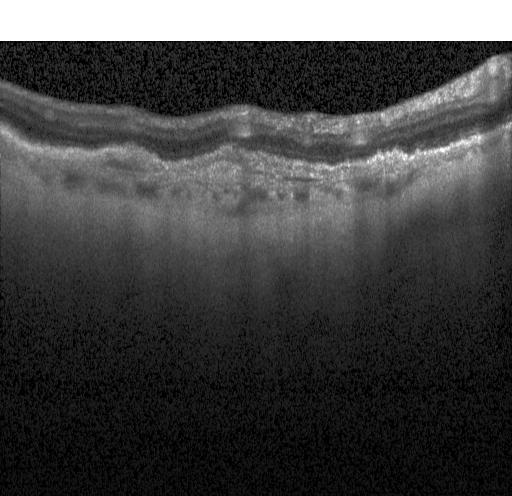

Spectral-domain optical coherence tomography; optical coherence tomography scan; through the macula.
Finding: a choroidal neovascular membrane.